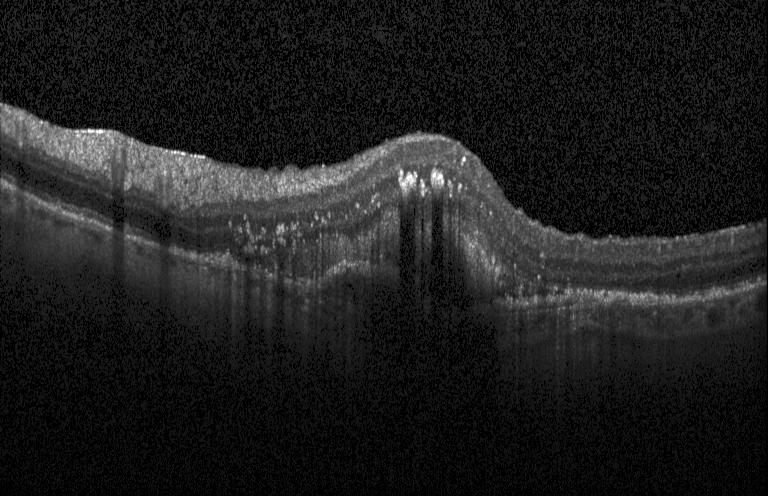

Acquired on a Heidelberg Spectralis; OCT B-scan
Impression: a choroidal neovascular membrane.